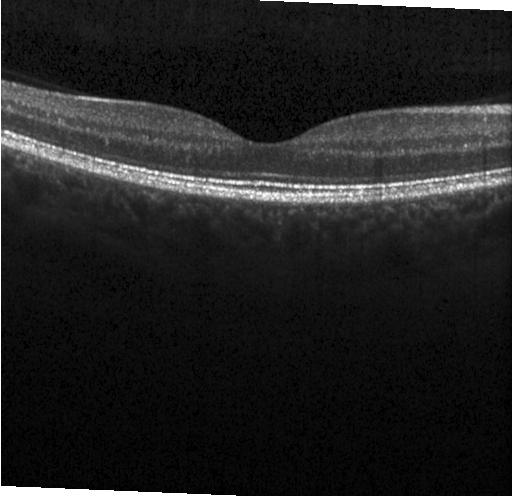 Retinal OCT B-scan, acquired on a Heidelberg Spectralis, spectral-domain OCT.
OCT finding: no choroidal neovascularization, diabetic macular edema, or drusen.